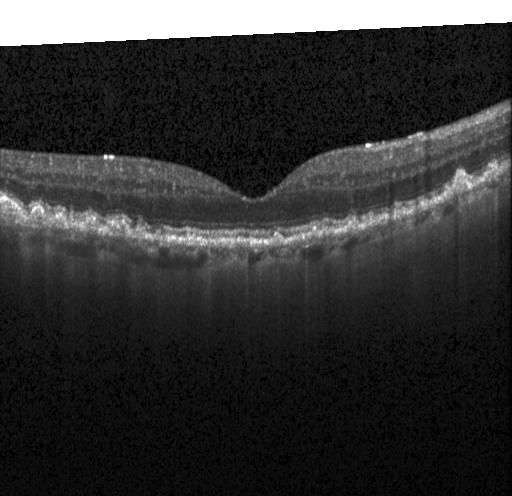

Optical coherence tomography scan. Horizontal scan through the fovea. Heidelberg Spectralis. Finding: sub-RPE drusenoid deposits.